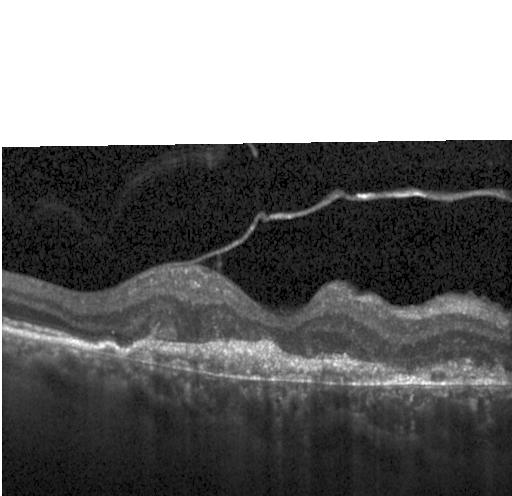 This B-scan demonstrates CNV.